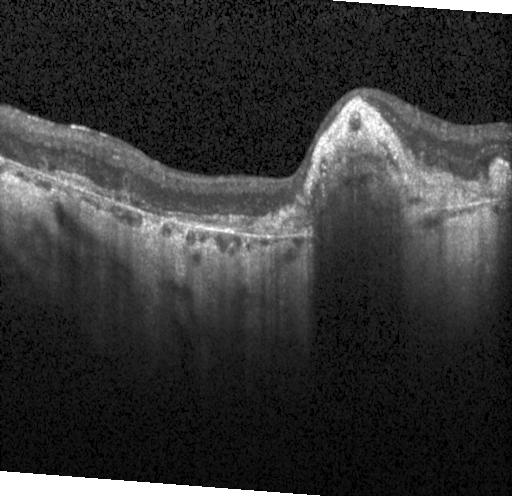 Horizontal scan through the fovea · spectral-domain OCT · retinal OCT cross-section · acquired on a Heidelberg Spectralis.
A choroidal neovascular membrane.